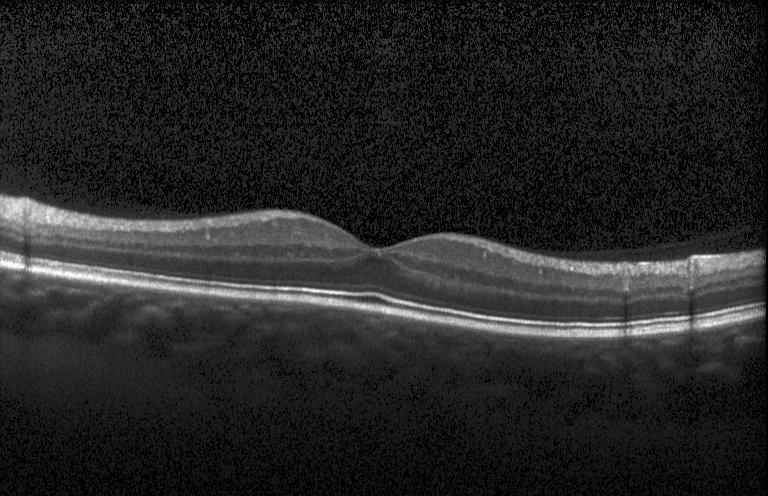 This B-scan demonstrates neither choroidal neovascularization, diabetic macular edema, nor drusen.